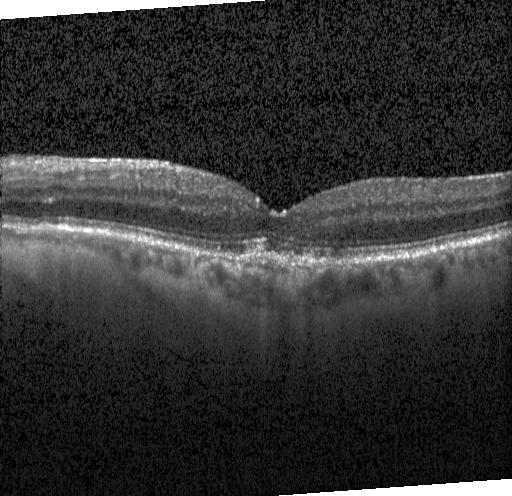 Spectral-domain OCT. Retinal OCT cross-section. Heidelberg Spectralis OCT system. Centered on the fovea — Impression: choroidal neovascularization.